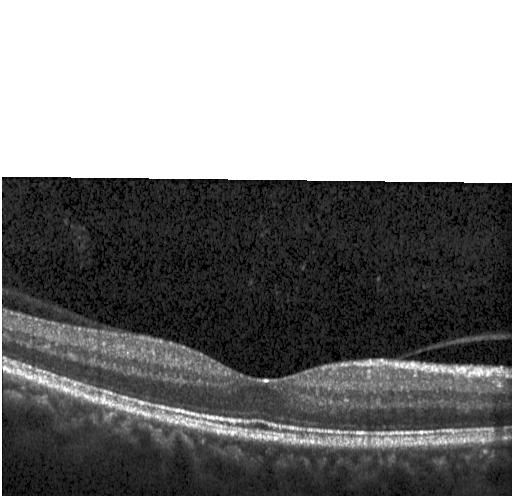 OCT line scan — Dx: no evidence of choroidal neovascularization, diabetic macular edema, or drusen.